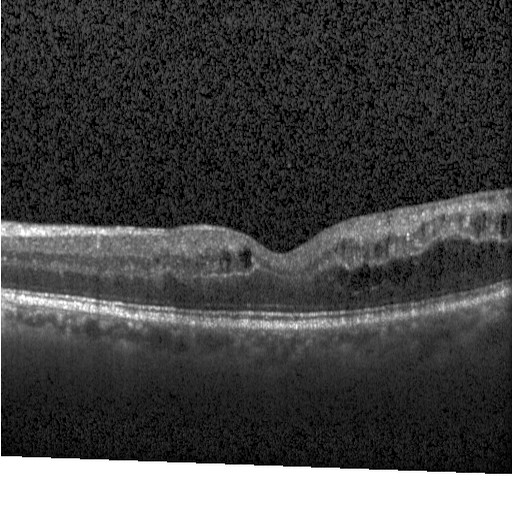
Instrument: Heidelberg Spectralis. Optical coherence tomography scan. Macular scan — Dx: DME.